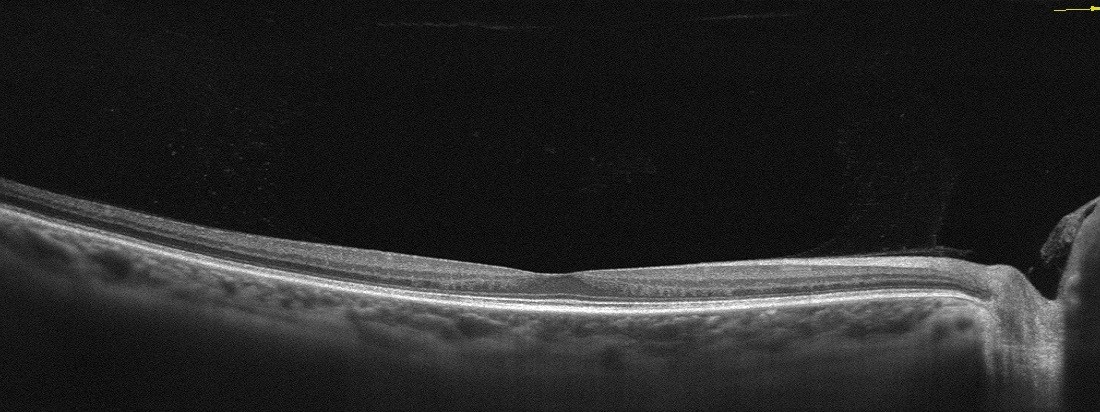

Fovea-centered. Retinal OCT B-scan.
Macular OCT: no evidence of AMD, DME, ERM, RAO, RVO, or VID.